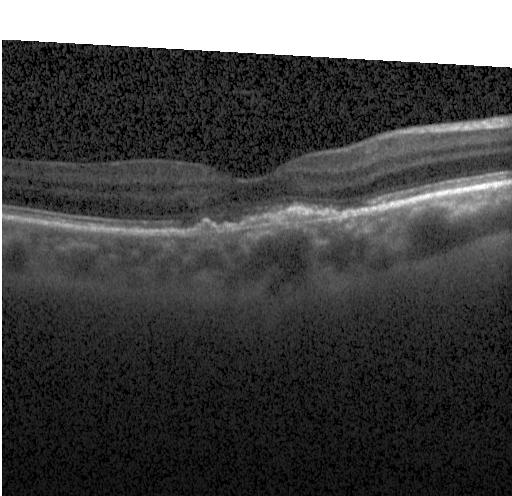

Spectral-domain OCT. OCT B-scan. Heidelberg Spectralis. Centered on the fovea — Diagnosis: a choroidal neovascular membrane.